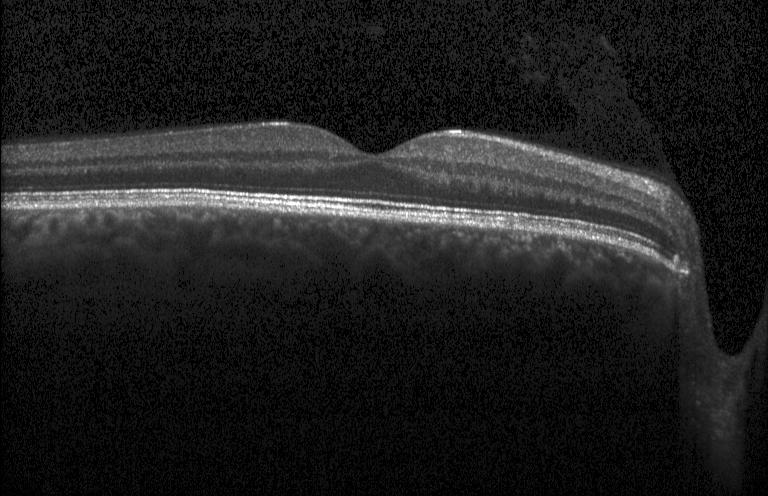
OCT line scan. Impression: no CNV, DME, or drusen.